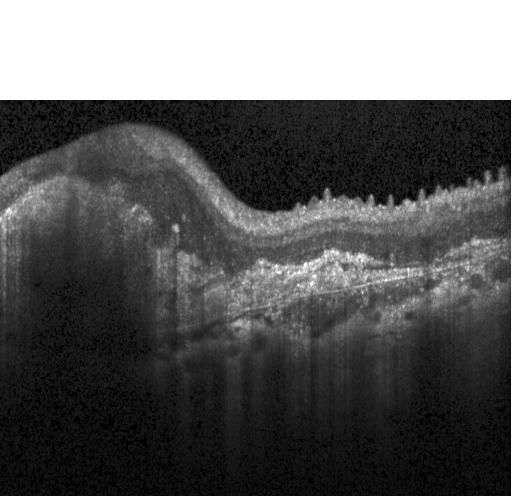 Heidelberg Spectralis OCT system · optical coherence tomography scan
Diagnosis: choroidal neovascularization (CNV).